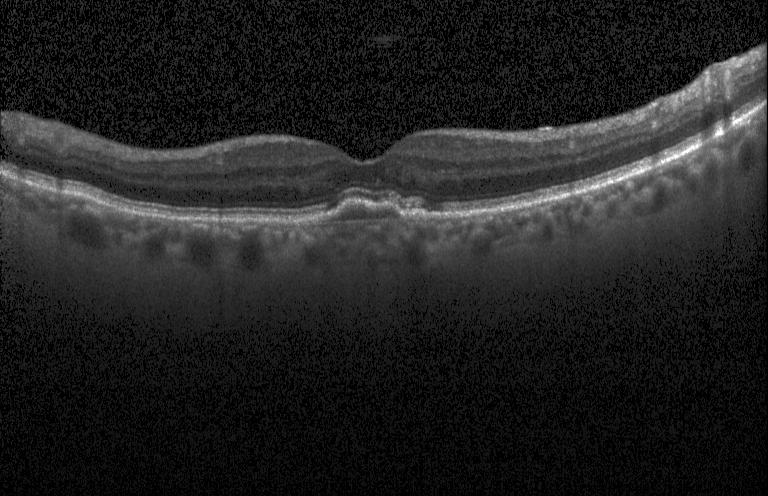 OCT B-scan.
Assessment: choroidal neovascularization.